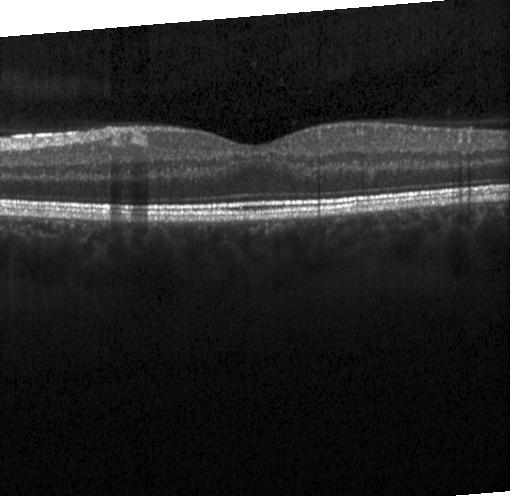
Dx: no evidence of choroidal neovascularization, diabetic macular edema, or drusen.